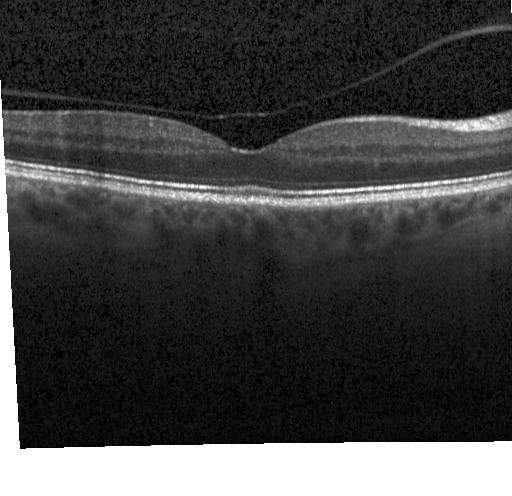
The scan shows no CNV, no DME, and no drusen.